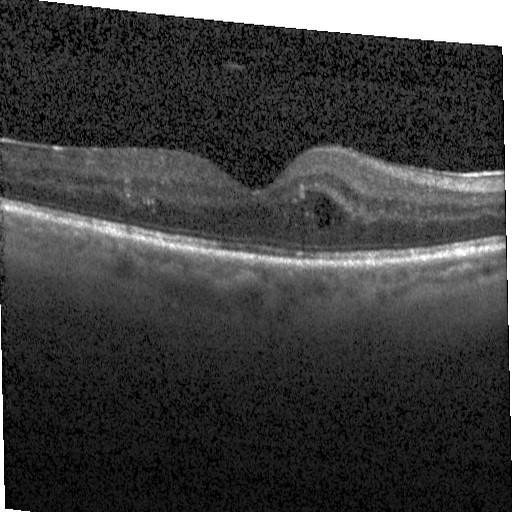

Retinal OCT B-scan; macular scan.
Diagnosis: diabetic macular edema.